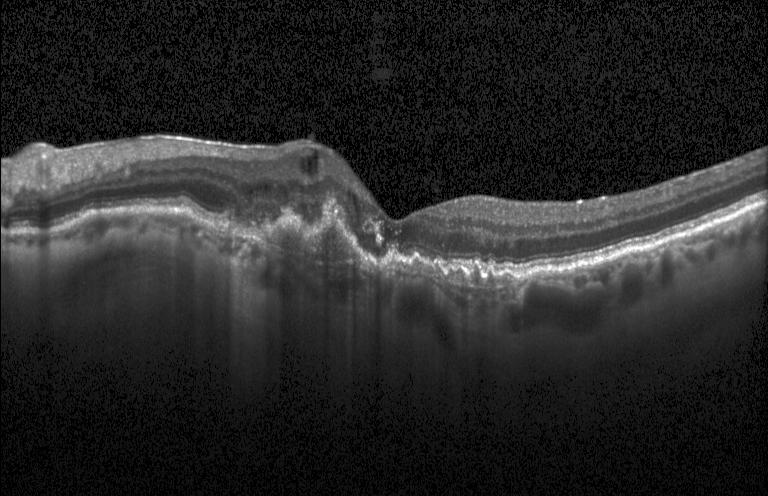

OCT scan showing choroidal neovascularization (CNV).